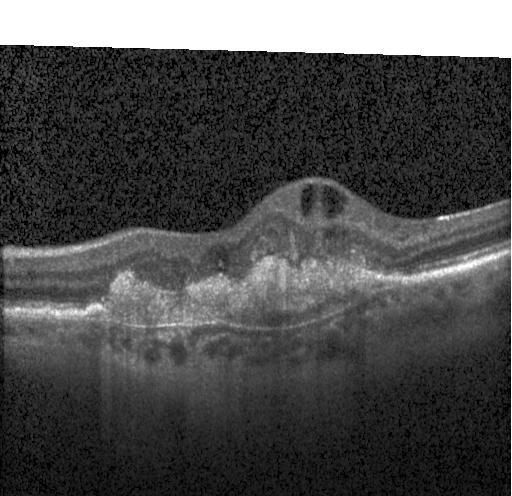

Retinal OCT B-scan. Instrument: Heidelberg Spectralis. Spectral-domain OCT — The scan shows choroidal neovascularization.